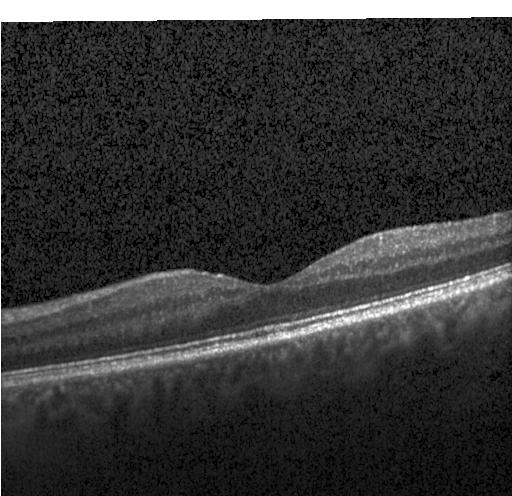

Retinal OCT B-scan, spectral-domain OCT, acquired on a Heidelberg Spectralis
The scan shows no evidence of choroidal neovascularization, diabetic macular edema, or drusen.